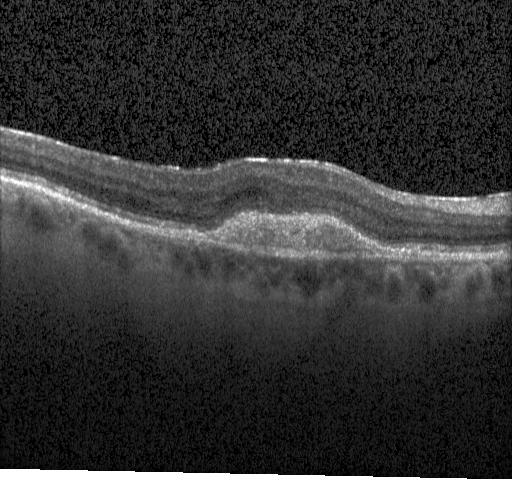

Finding: a choroidal neovascular membrane.